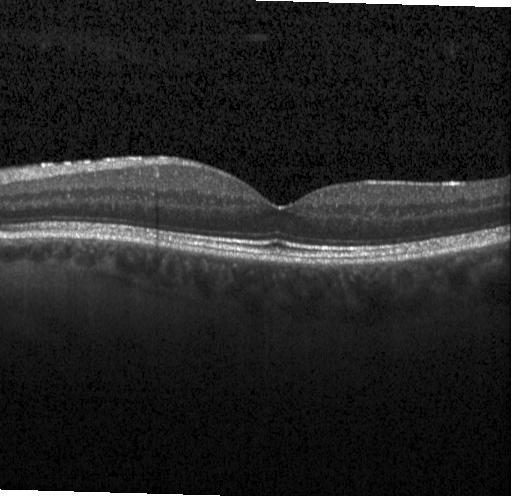
OCT B-scan showing no evidence of choroidal neovascularization, diabetic macular edema, or drusen.